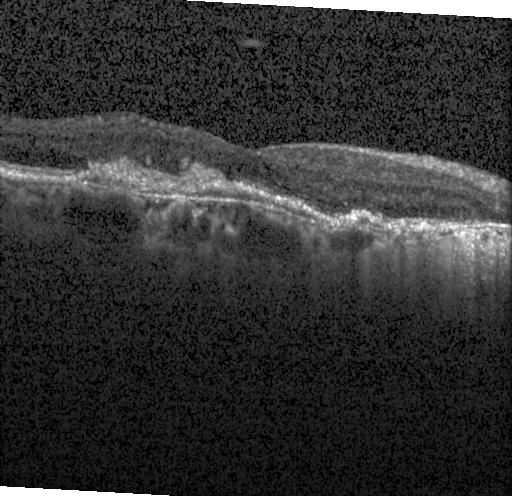

Retinal OCT B-scan; Heidelberg Spectralis
The scan shows choroidal neovascularization (CNV).